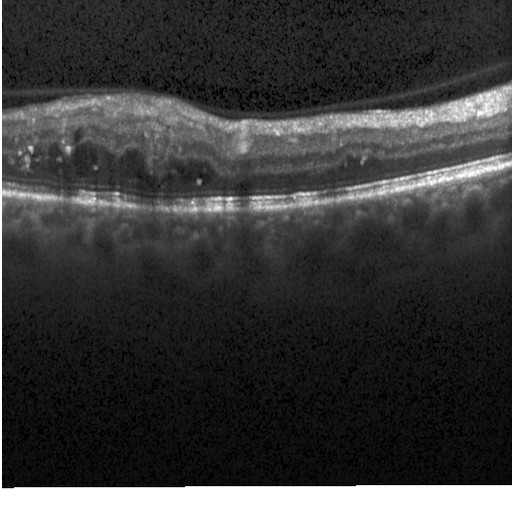
Heidelberg Spectralis, OCT line scan — OCT finding: diabetic macular edema (DME).